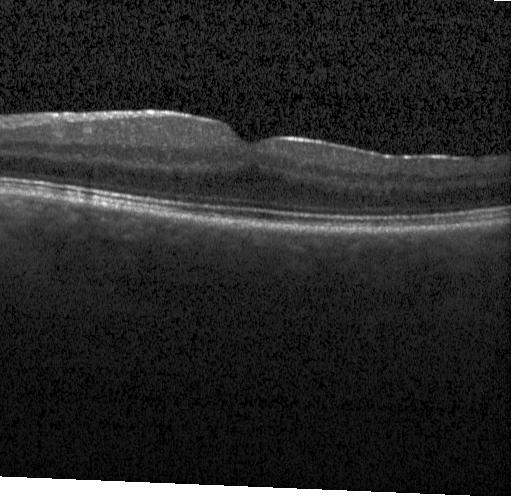
OCT finding: no evidence of choroidal neovascularization, diabetic macular edema, or drusen.